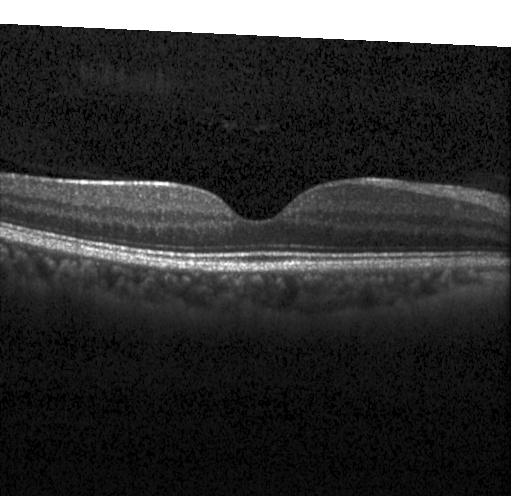

No CNV, no DME, and no drusen.